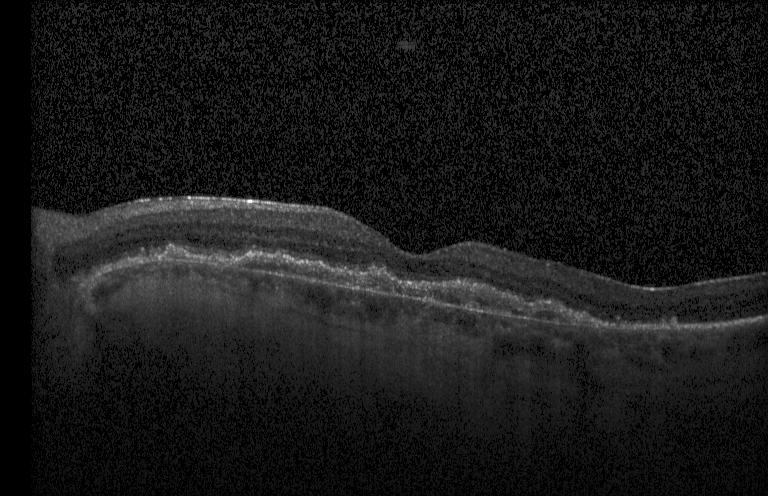
OCT B-scan showing CNV.